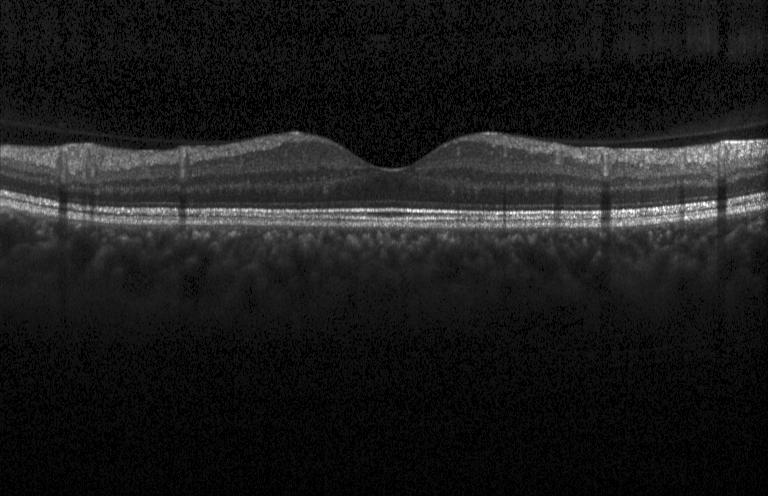

Spectral-domain OCT B-scan: neither CNV, DME, nor drusen.